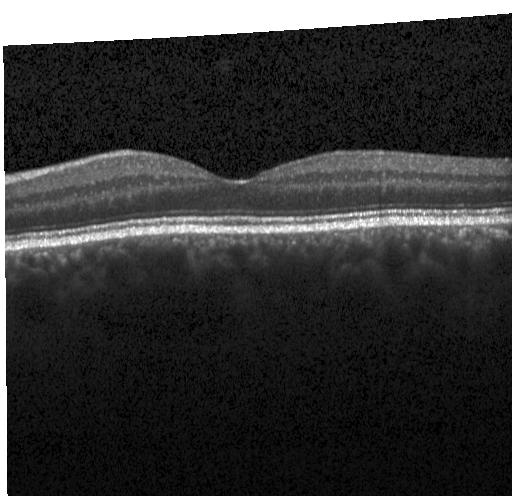
Retinal OCT cross-section · Heidelberg Spectralis · SD-OCT — No evidence of choroidal neovascularization, diabetic macular edema, or drusen.